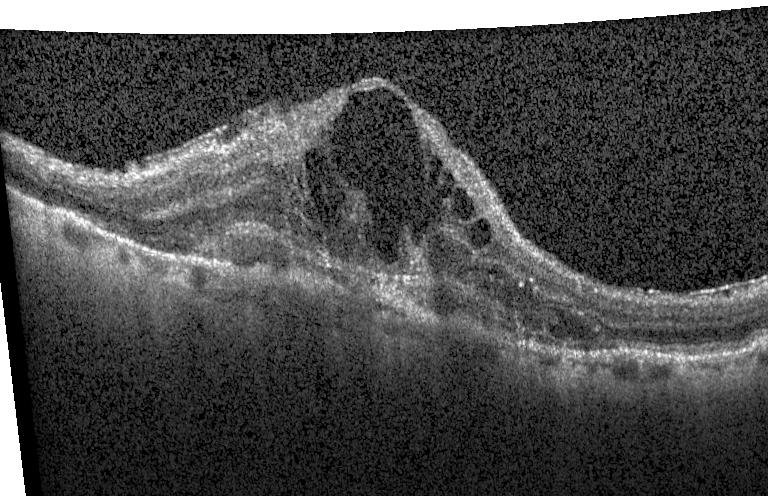
Retinal OCT cross-section, spectral-domain OCT
Impression: choroidal neovascularization.